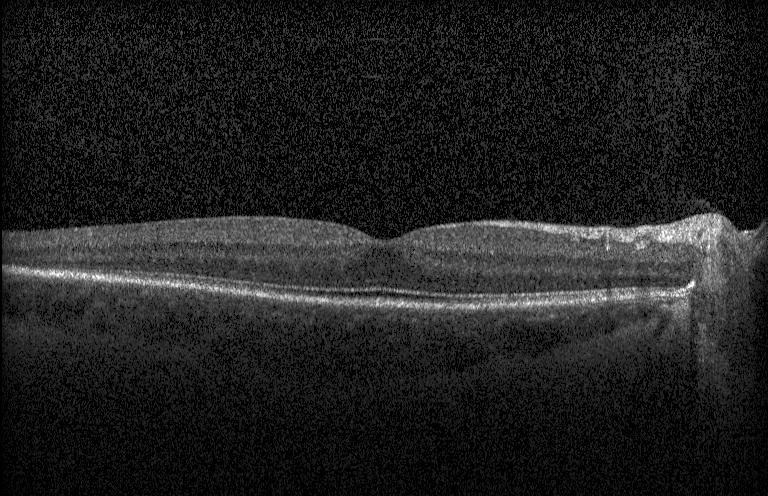 Diagnosis: no choroidal neovascularization, no diabetic macular edema, and no drusen.